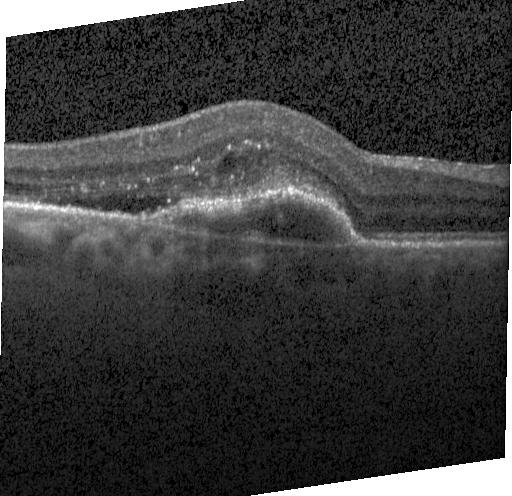

Macular scan. Instrument: Heidelberg Spectralis. OCT line scan. Finding: CNV.